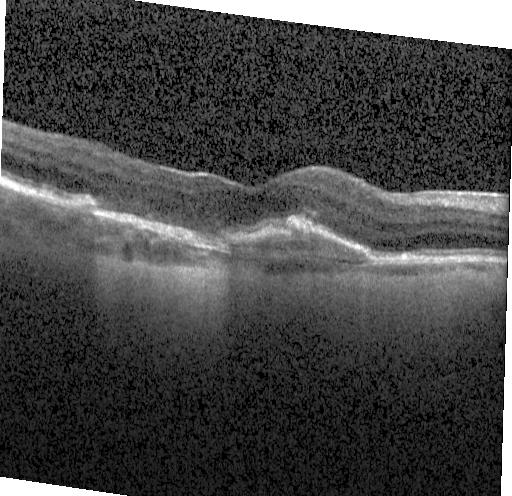

Retinal OCT cross-section. Instrument: Heidelberg Spectralis. SD-OCT.
This B-scan demonstrates a choroidal neovascular membrane.